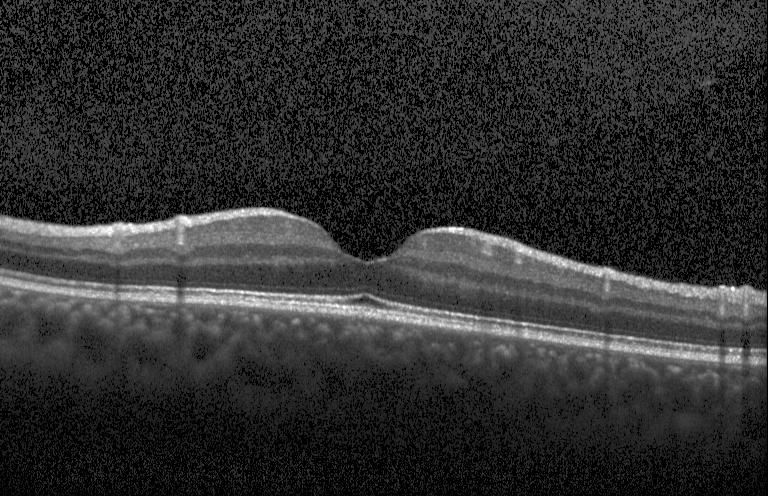
OCT finding: neither choroidal neovascularization, diabetic macular edema, nor drusen.